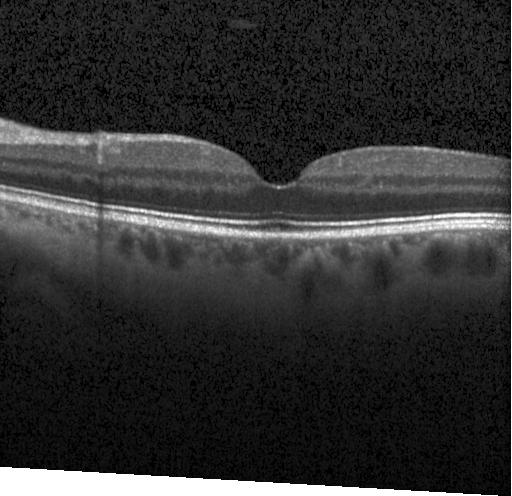

Optical coherence tomography scan · Heidelberg Spectralis OCT system — Impression: no evidence of CNV, DME, or drusen.